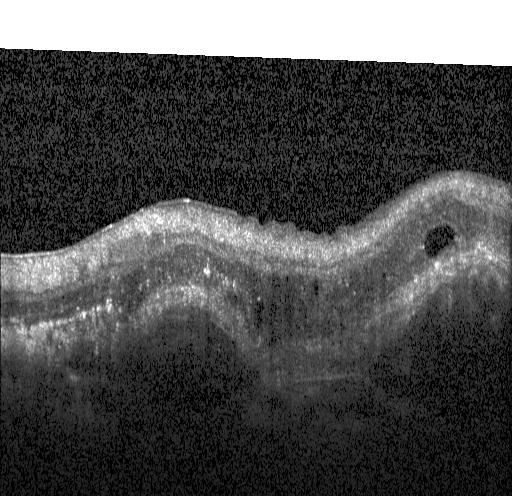 Macular scan. Retinal OCT cross-section.
Finding: choroidal neovascularization.